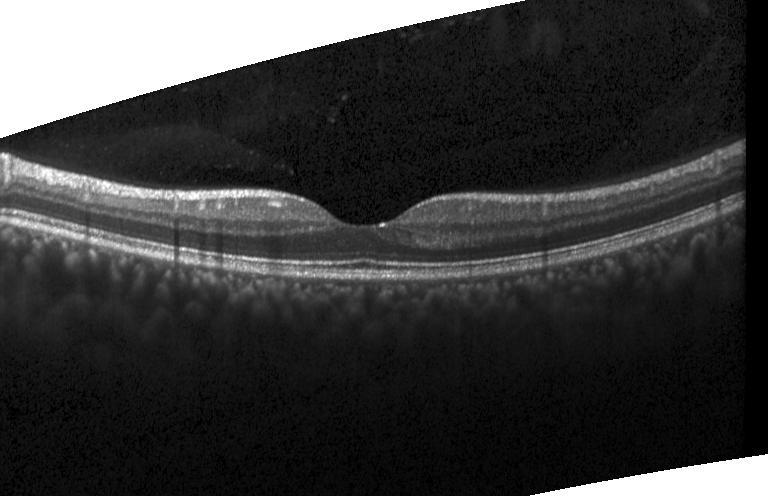

This B-scan demonstrates no evidence of CNV, DME, or drusen.